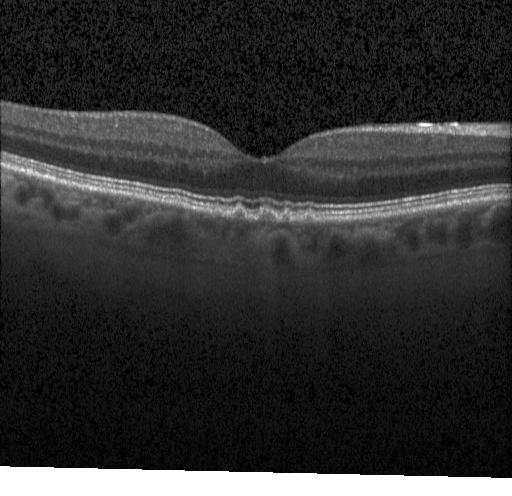
Retinal OCT cross-section — Impression: multiple drusen.